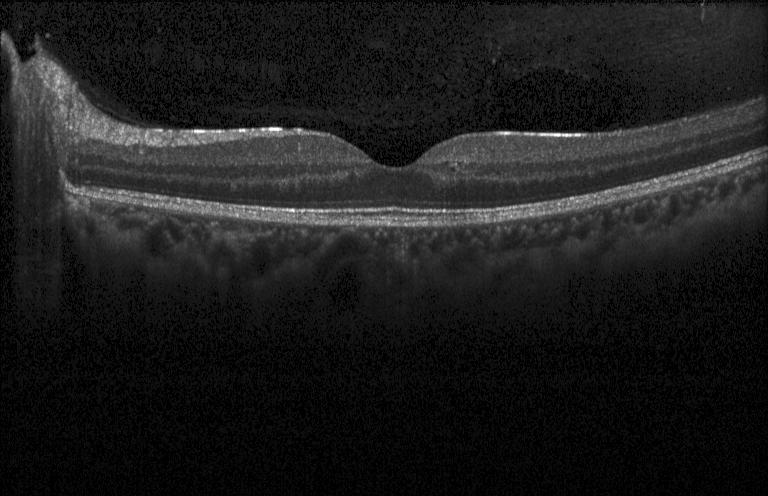

OCT scan showing no CNV, no DME, and no drusen.